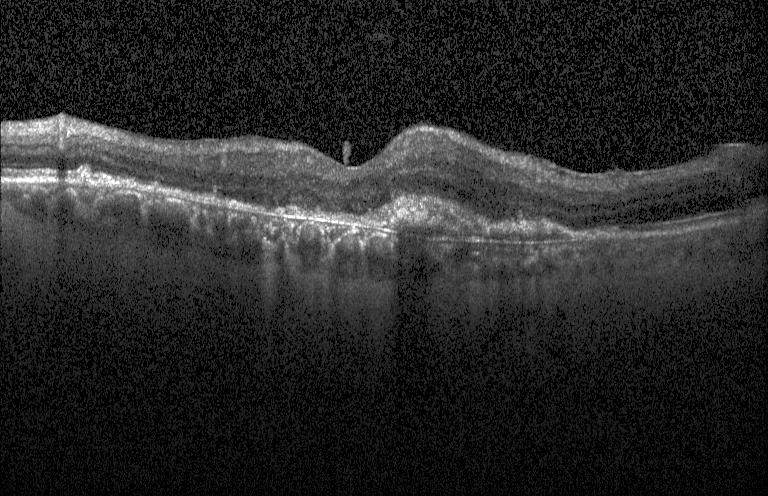

OCT scan showing a choroidal neovascular membrane.